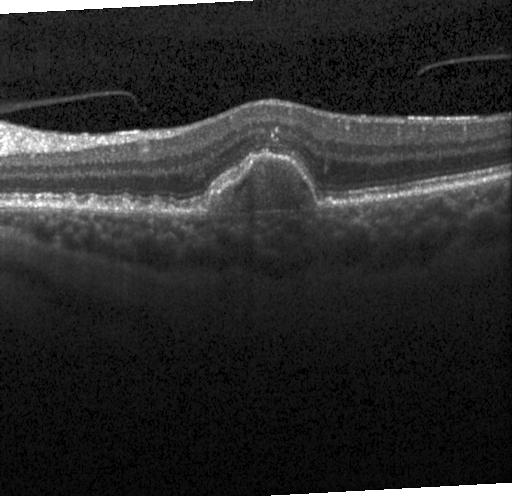 The scan shows choroidal neovascularization (CNV).